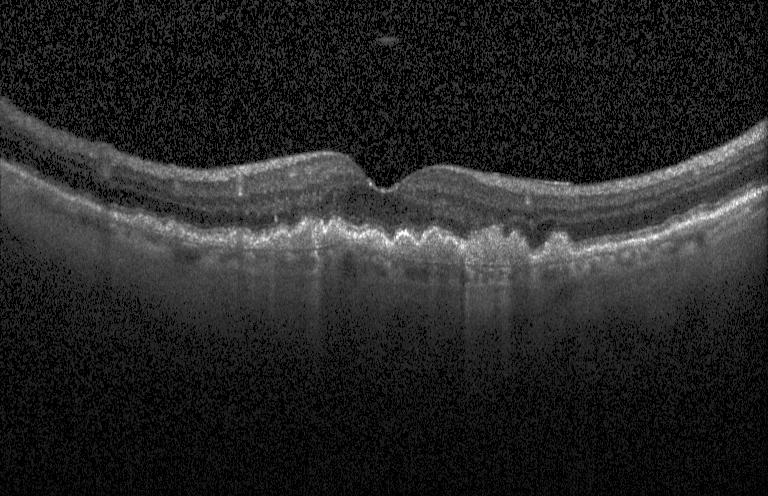

The scan shows multiple drusen.